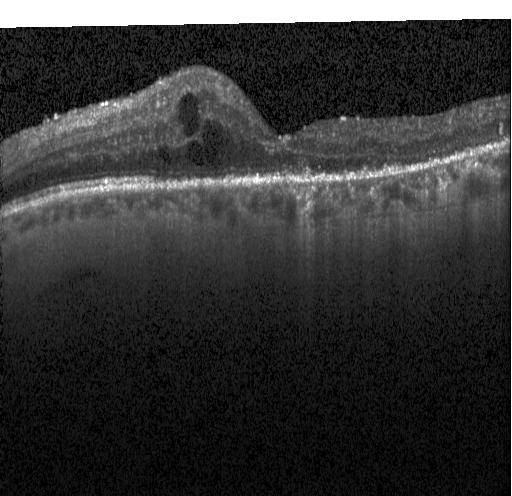

Macular OCT: diabetic macular edema (DME).